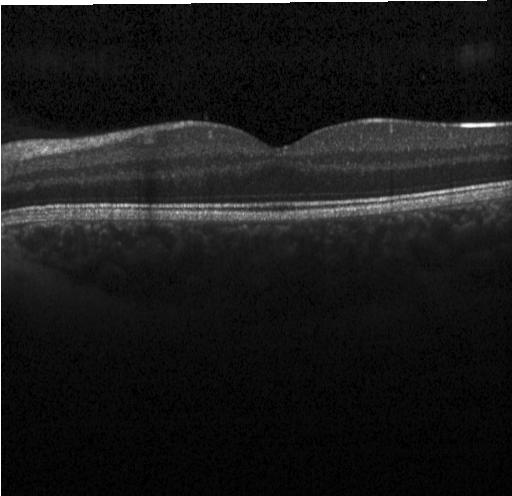
Diagnosis: no choroidal neovascularization, no diabetic macular edema, and no drusen.